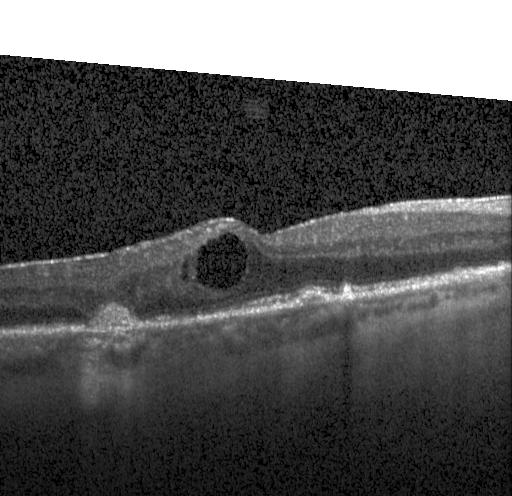

OCT B-scan showing a choroidal neovascular membrane.